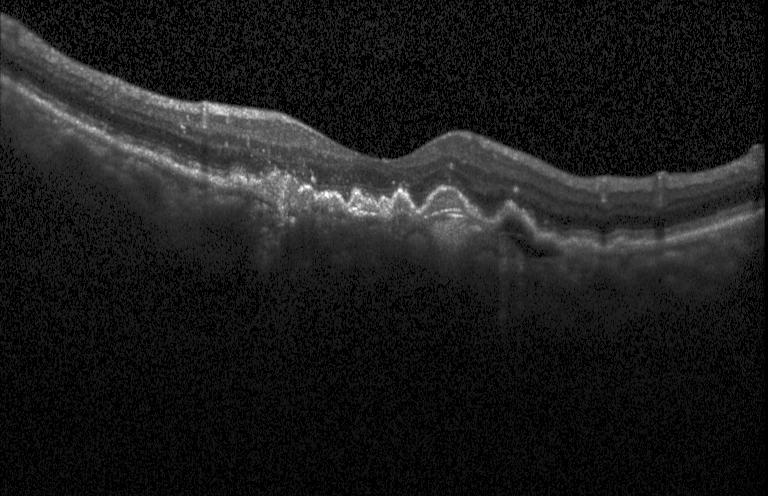
Impression: a choroidal neovascular membrane.